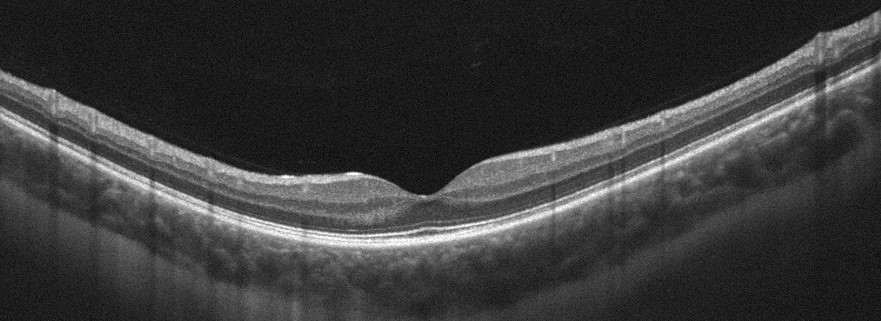
Optovue Avanti RTVue XR. OCT line scan. Diagnosis: absence of AMD, DME, ERM, RAO, RVO, and vitreomacular interface disease.